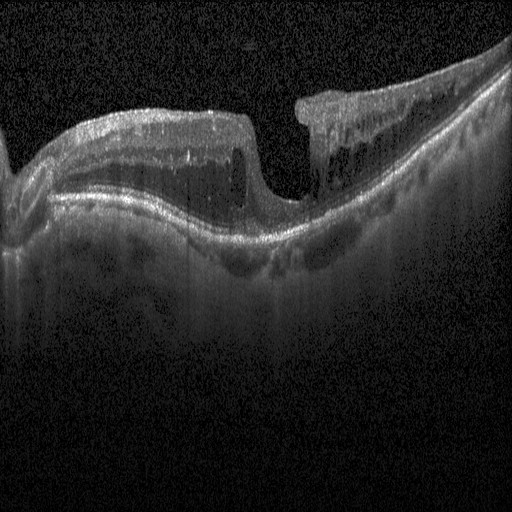 The scan shows DME.